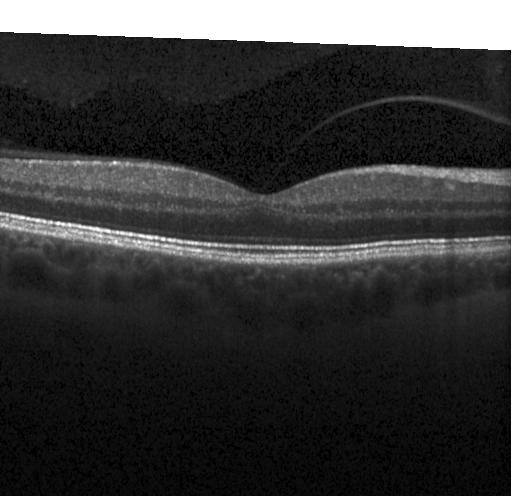

Diagnosis: no choroidal neovascularization, no diabetic macular edema, and no drusen.